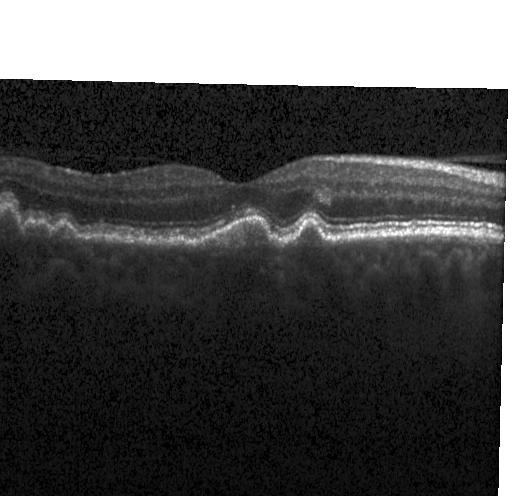

Retinal OCT cross-section showing drusen.